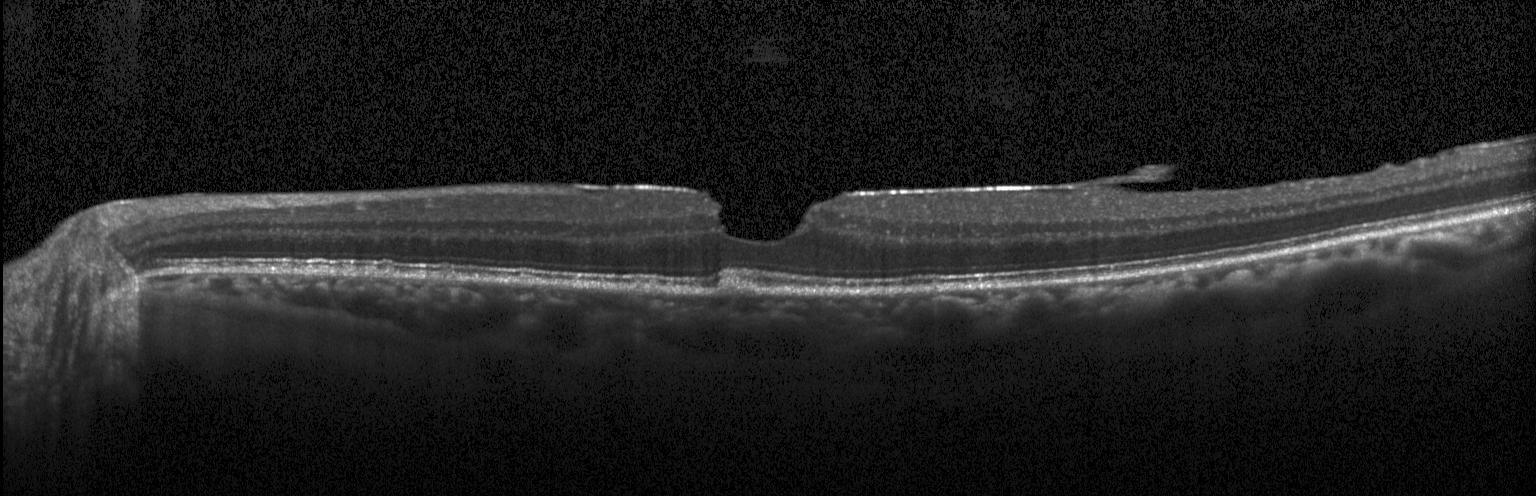 Acquired on a Heidelberg Spectralis, OCT B-scan. Dx: sub-RPE drusenoid deposits.